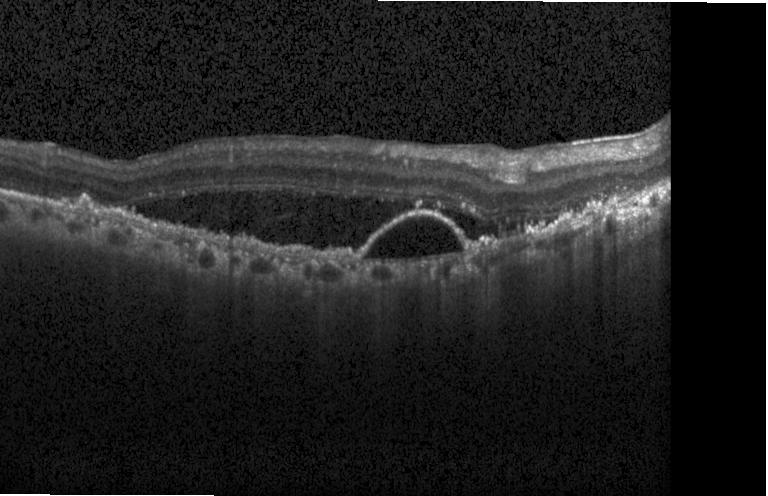

Assessment: a choroidal neovascular membrane.